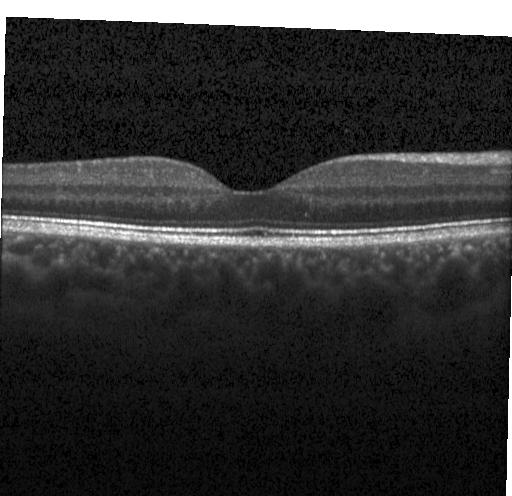

Retinal OCT cross-section showing neither choroidal neovascularization, diabetic macular edema, nor drusen.